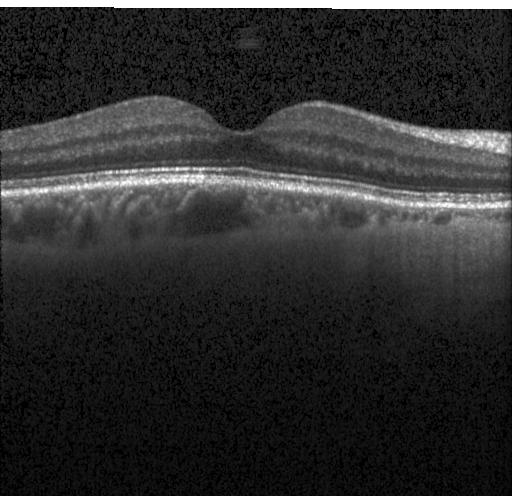
Spectral-domain OCT · acquired on a Heidelberg Spectralis · optical coherence tomography B-scan · macular scan
Diagnosis: no evidence of choroidal neovascularization, diabetic macular edema, or drusen.